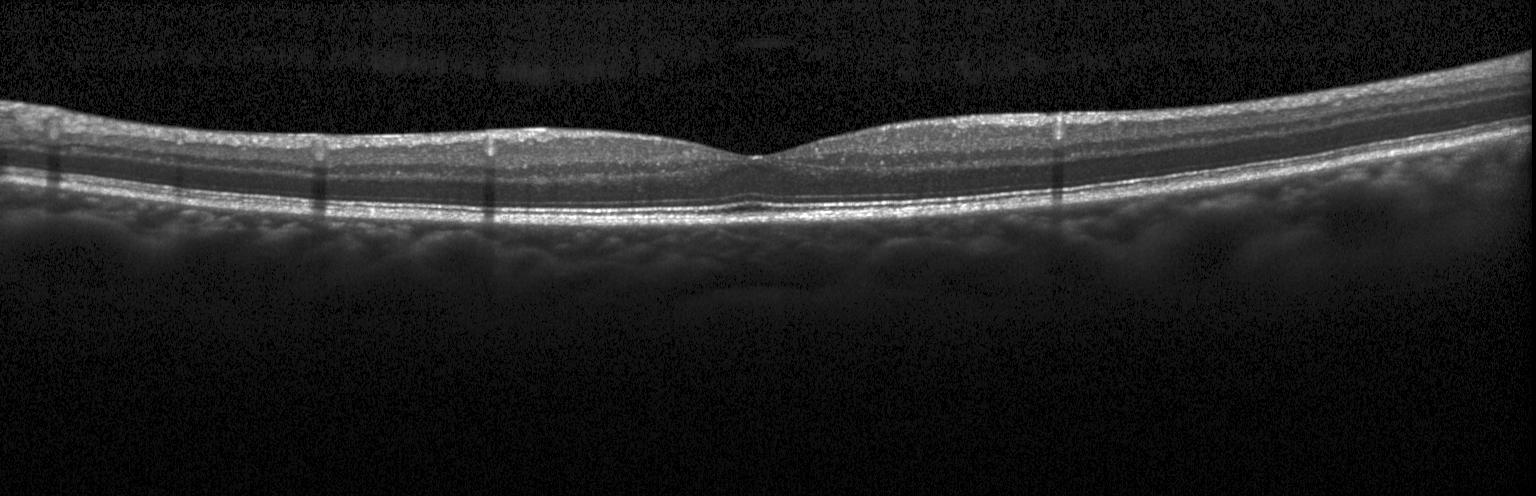
OCT line scan — Impression: no choroidal neovascularization, diabetic macular edema, or drusen.